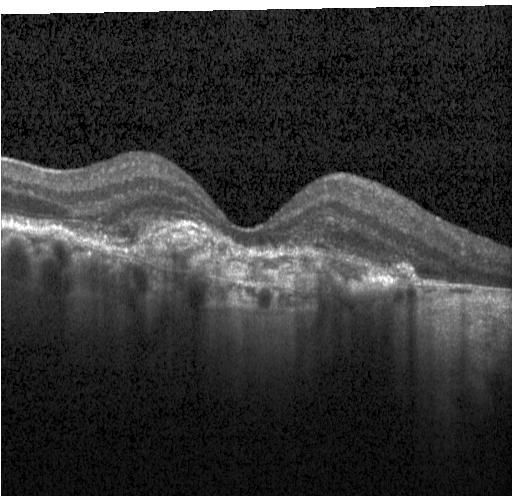

Acquired on a Heidelberg Spectralis. Optical coherence tomography scan. Macular scan.
Finding: choroidal neovascularization.